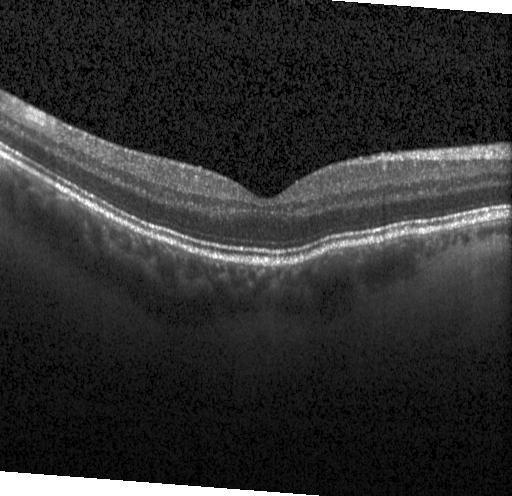

Spectral-domain optical coherence tomography · instrument: Heidelberg Spectralis · retinal OCT B-scan — Diagnosis: no evidence of choroidal neovascularization, diabetic macular edema, or drusen.